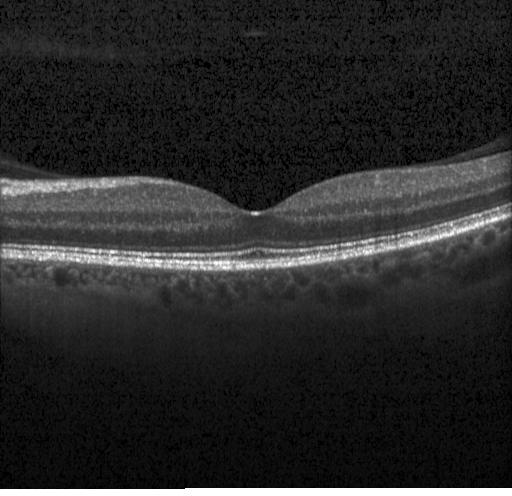
Finding: no evidence of CNV, DME, or drusen.